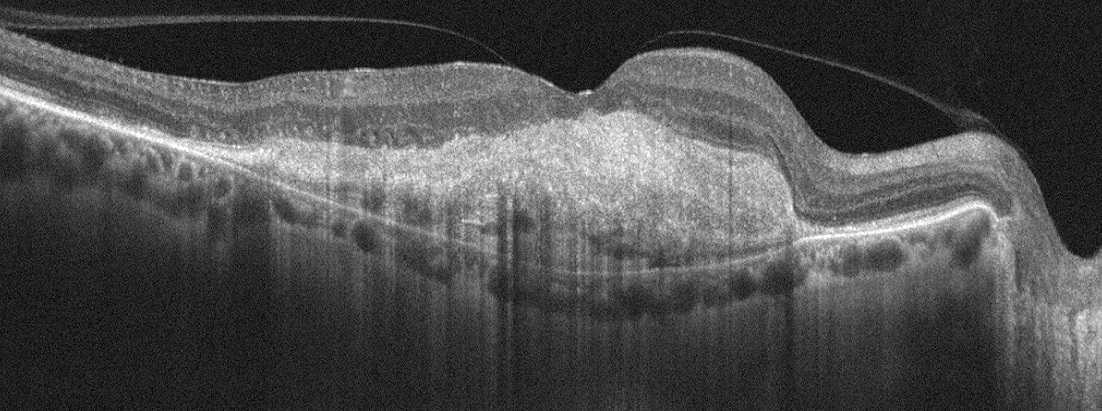

OCT B-scan; macular scan — Impression: age-related macular degeneration.